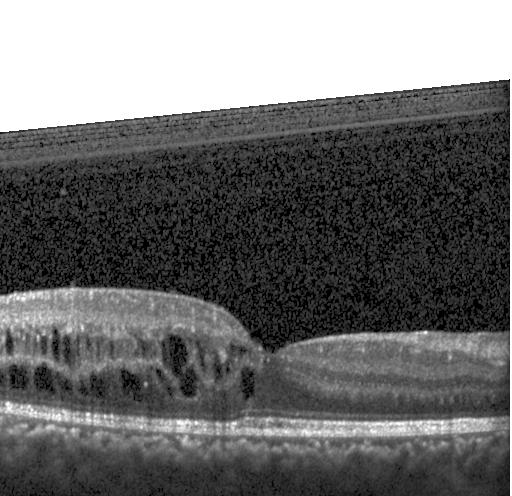
Optical coherence tomography scan. Fovea-centered. SD-OCT. Instrument: Heidelberg Spectralis. Impression: diabetic macular edema.